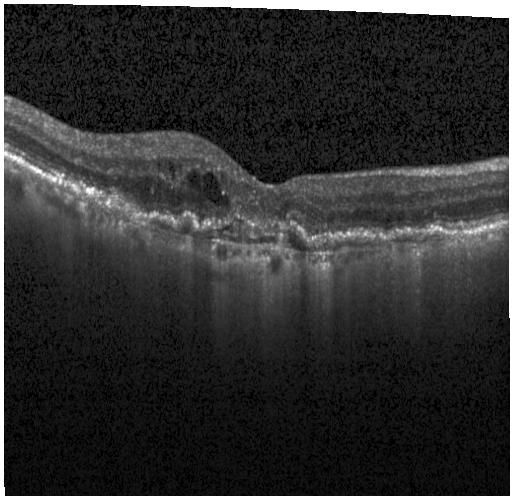

OCT line scan — Macular OCT: a choroidal neovascular membrane.